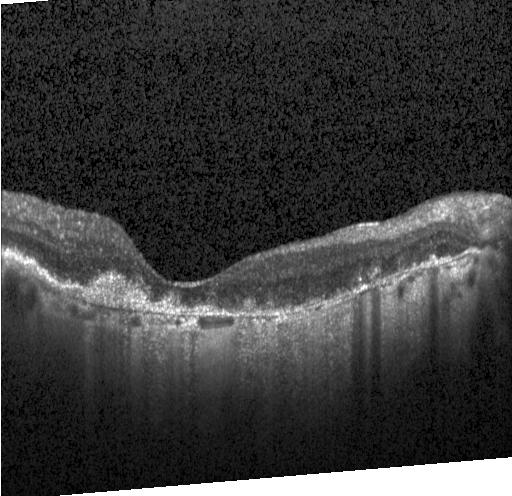
A choroidal neovascular membrane.